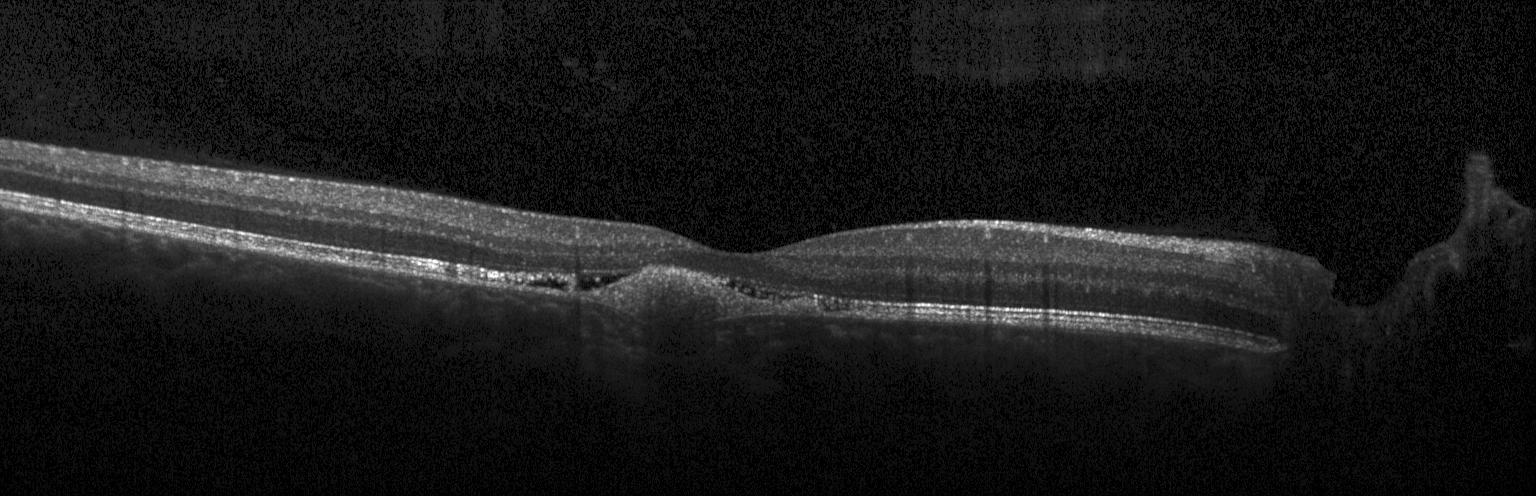 OCT B-scan showing choroidal neovascularization (CNV).